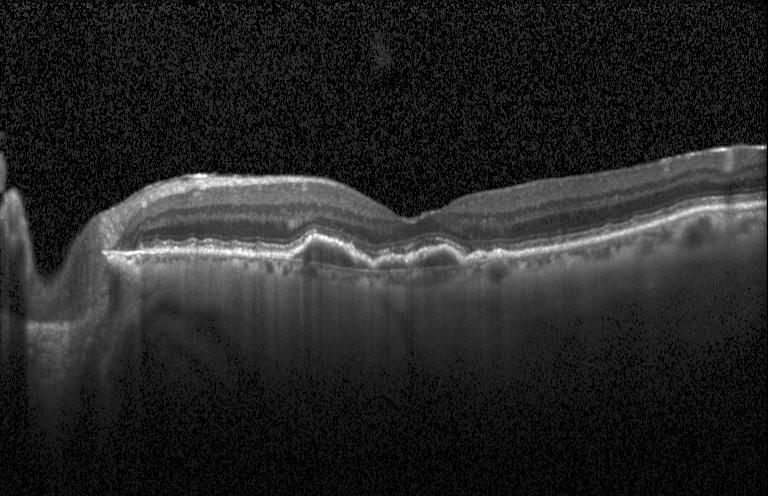 Retinal OCT cross-section showing CNV.